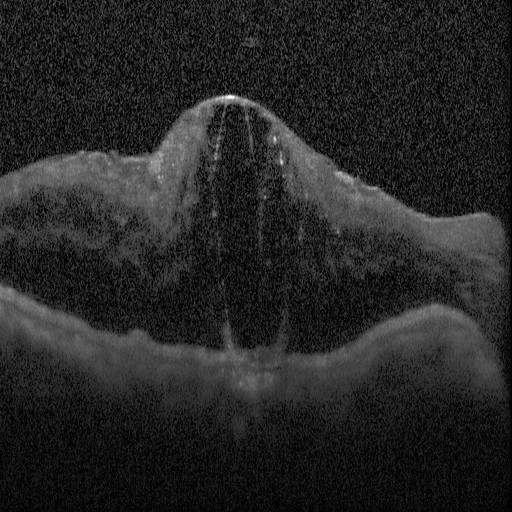 Finding: diabetic macular edema.